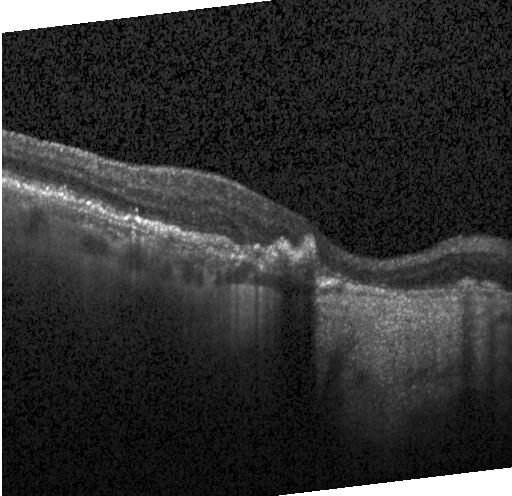

Instrument: Heidelberg Spectralis; OCT line scan
Dx: choroidal neovascularization (CNV).